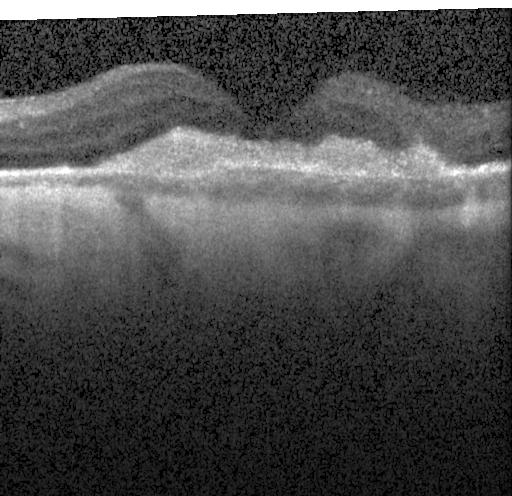
OCT B-scan — Assessment: choroidal neovascularization.